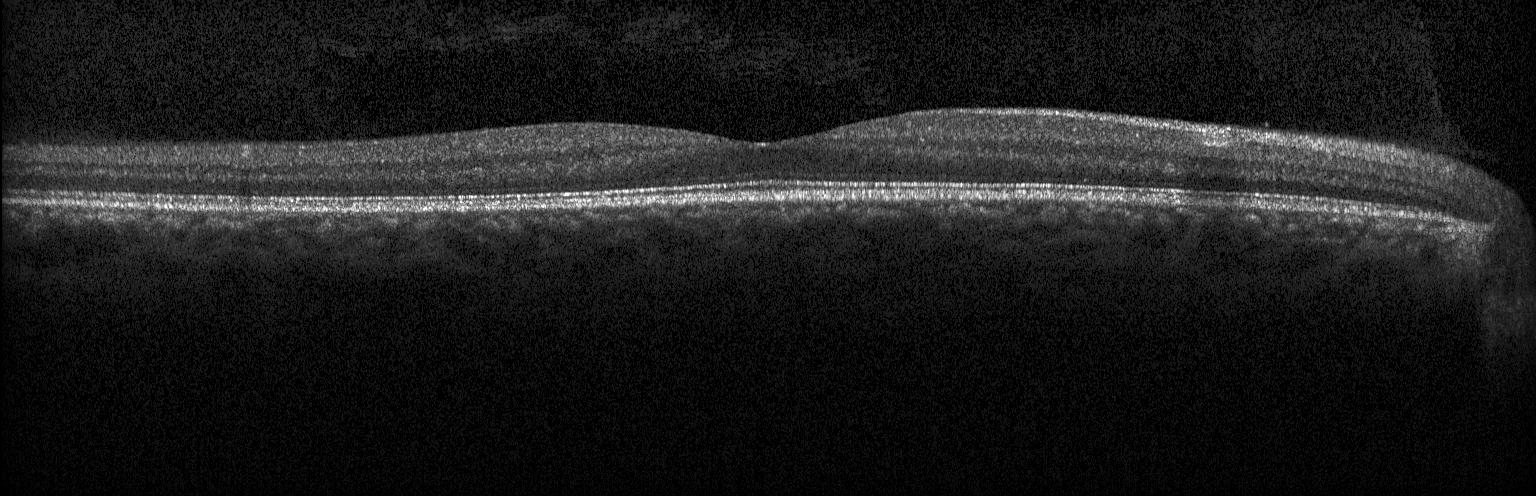
SD-OCT. Heidelberg Spectralis. OCT line scan. Through the macula. OCT finding: no choroidal neovascularization, diabetic macular edema, or drusen.